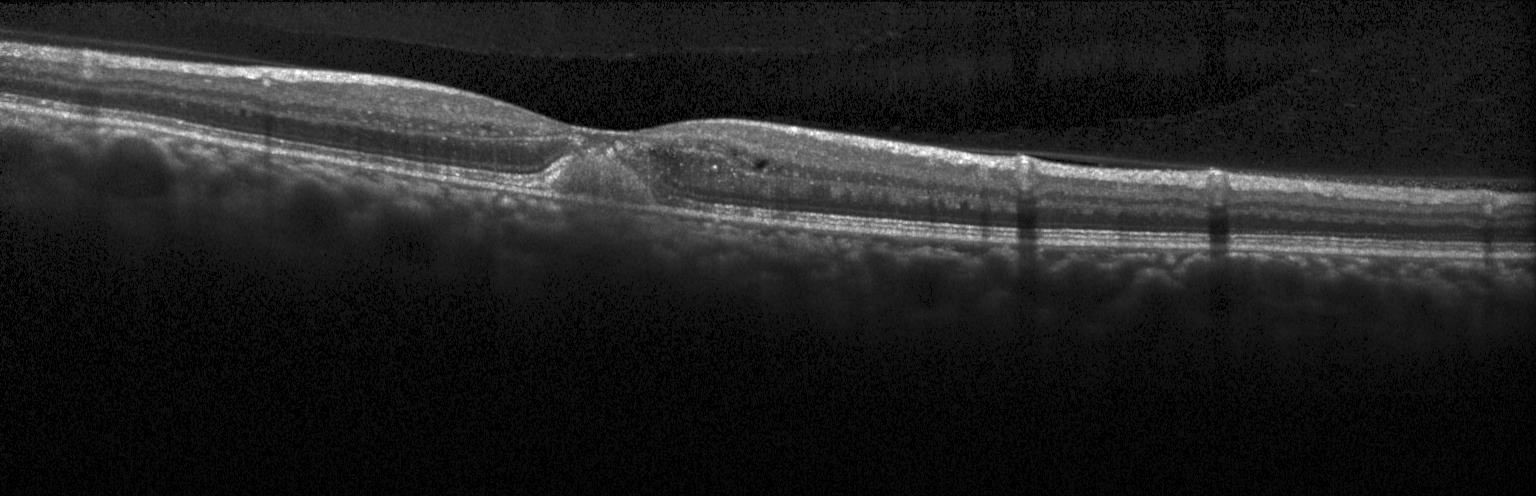 Retinal OCT cross-section · spectral-domain optical coherence tomography.
OCT finding: CNV.